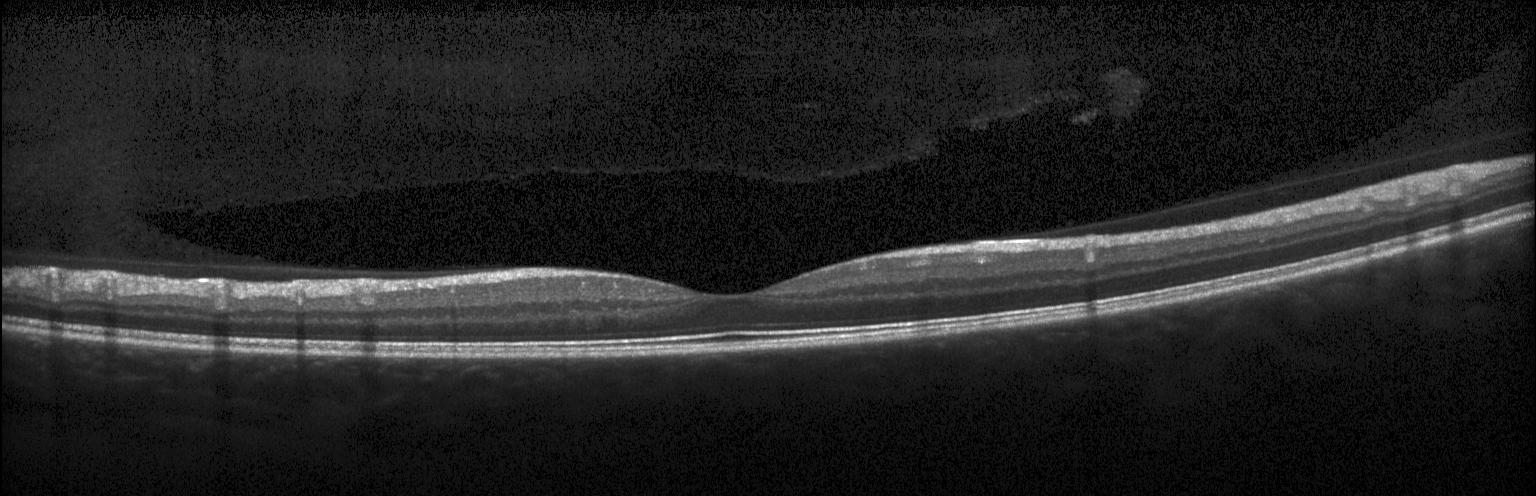
Diagnosis: no CNV, DME, or drusen.